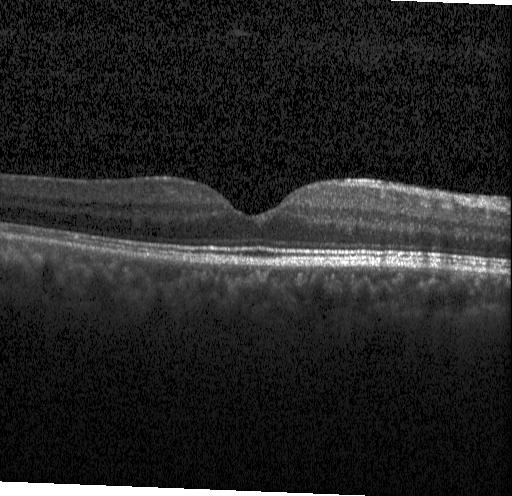
Macular OCT demonstrating no choroidal neovascularization, no diabetic macular edema, and no drusen.